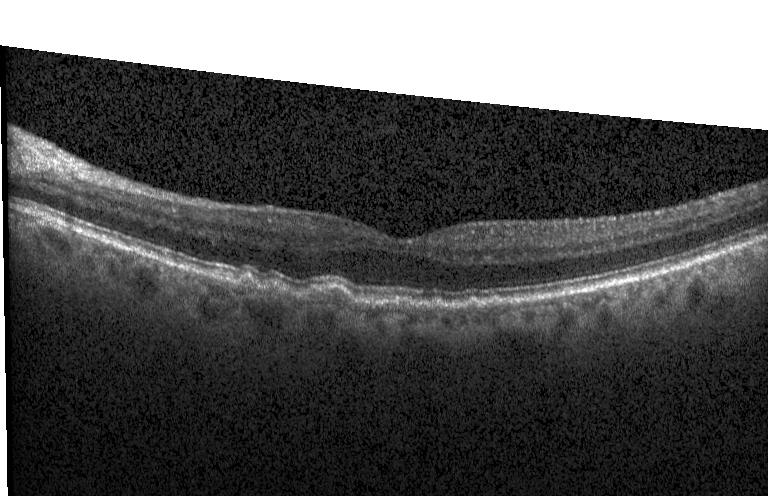
Heidelberg Spectralis · through the macula · optical coherence tomography scan · spectral-domain optical coherence tomography — Dx: multiple drusen.